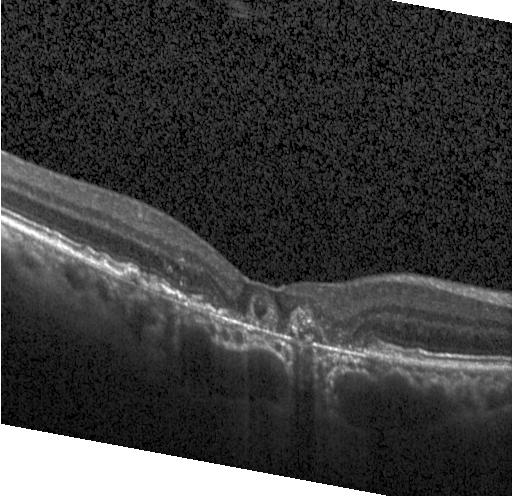

Impression: a choroidal neovascular membrane.